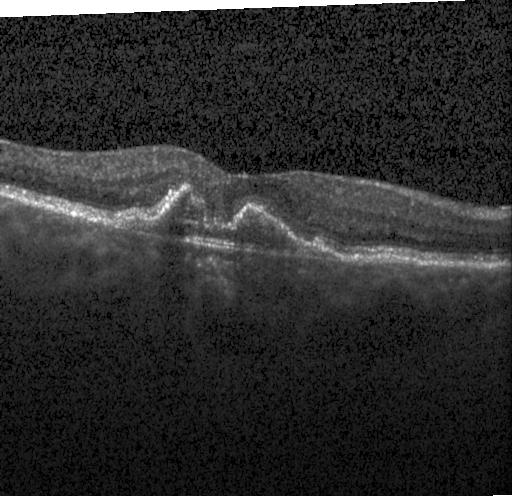
Assessment: a choroidal neovascular membrane.